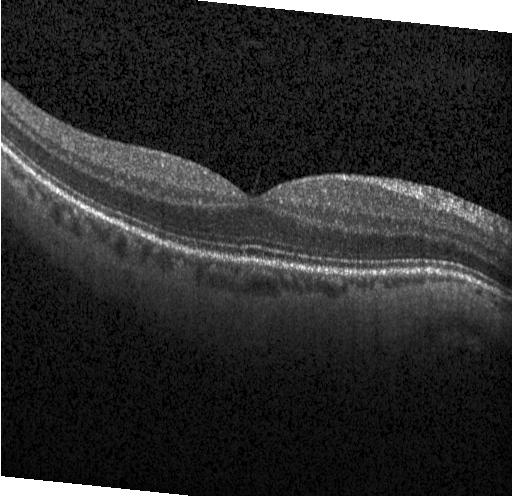
Through the macula, spectral-domain optical coherence tomography, optical coherence tomography scan.
Diagnosis: no evidence of choroidal neovascularization, diabetic macular edema, or drusen.